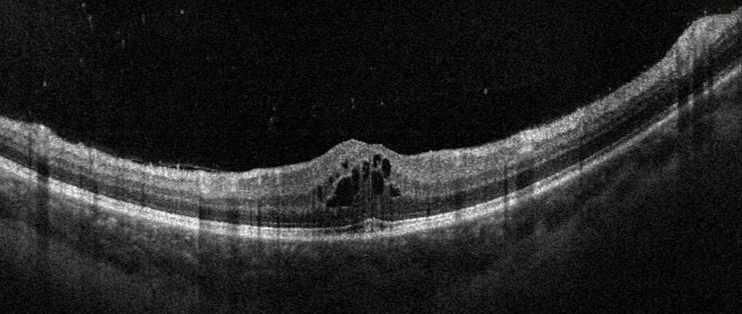 OCT B-scan. Instrument: Optovue Avanti RTVue XR. Through the macula.
Impression: diabetic macular edema.